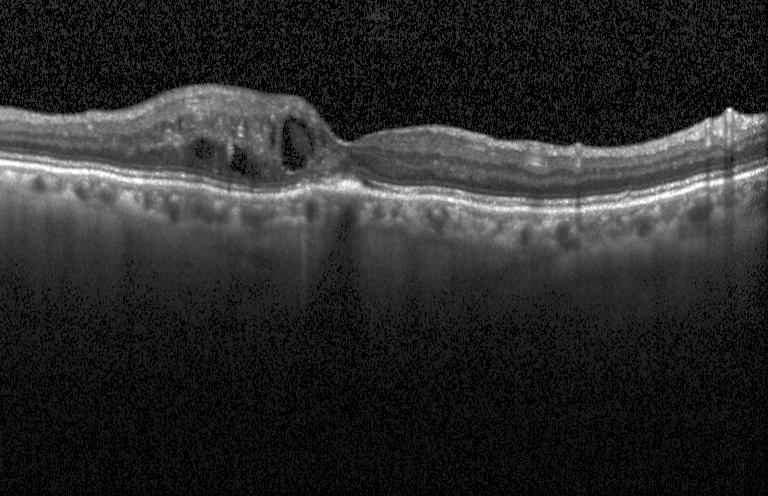 Instrument: Heidelberg Spectralis, horizontal scan through the fovea, optical coherence tomography B-scan, spectral-domain optical coherence tomography — Macular OCT: diabetic macular edema (DME).